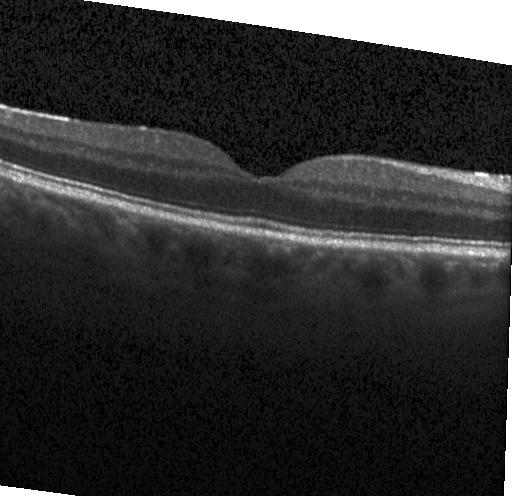
Heidelberg Spectralis OCT system, OCT line scan, spectral-domain OCT, centered on the fovea
This B-scan demonstrates no choroidal neovascularization, no diabetic macular edema, and no drusen.